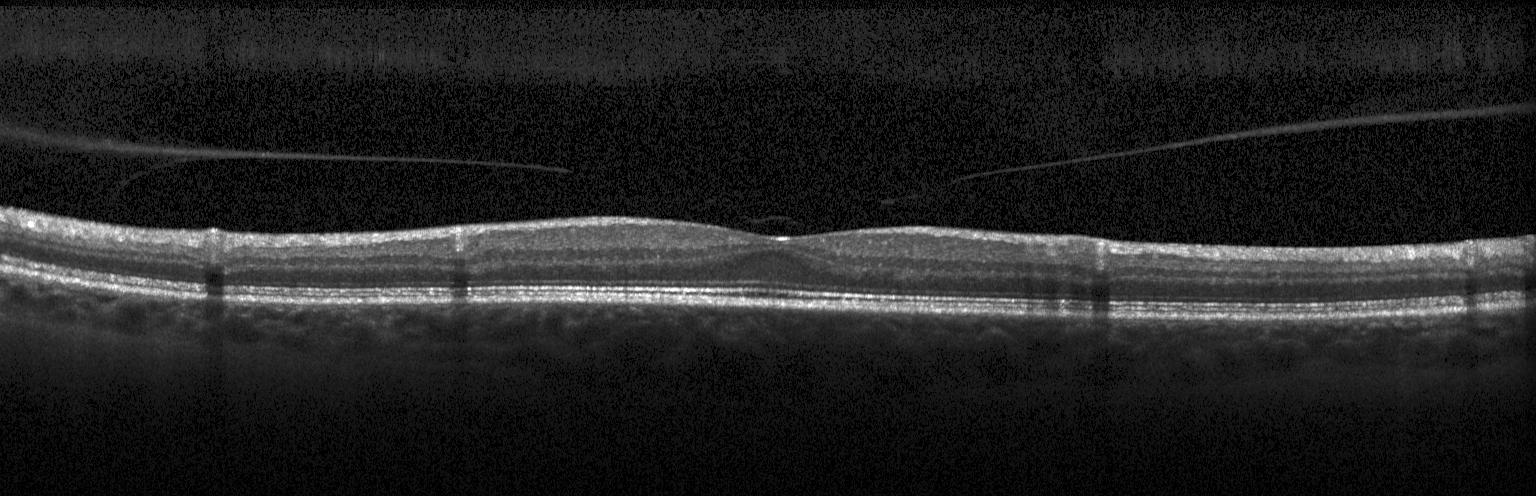

Impression: neither choroidal neovascularization, diabetic macular edema, nor drusen.